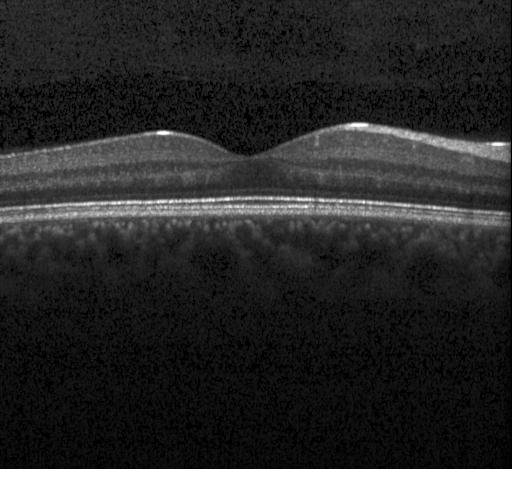
Retinal OCT B-scan
Finding: no choroidal neovascularization, diabetic macular edema, or drusen.